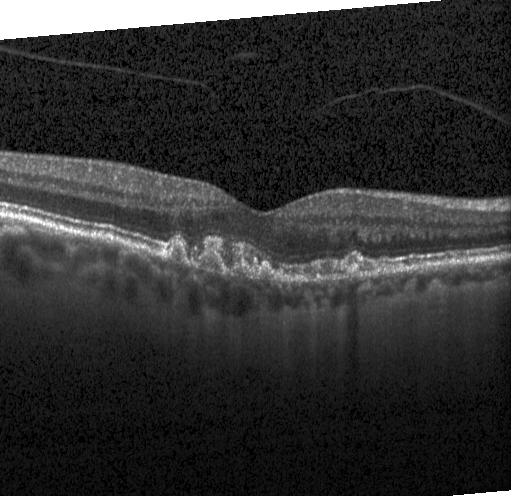 Spectral-domain OCT · optical coherence tomography scan · instrument: Heidelberg Spectralis · fovea-centered — Impression: a choroidal neovascular membrane.